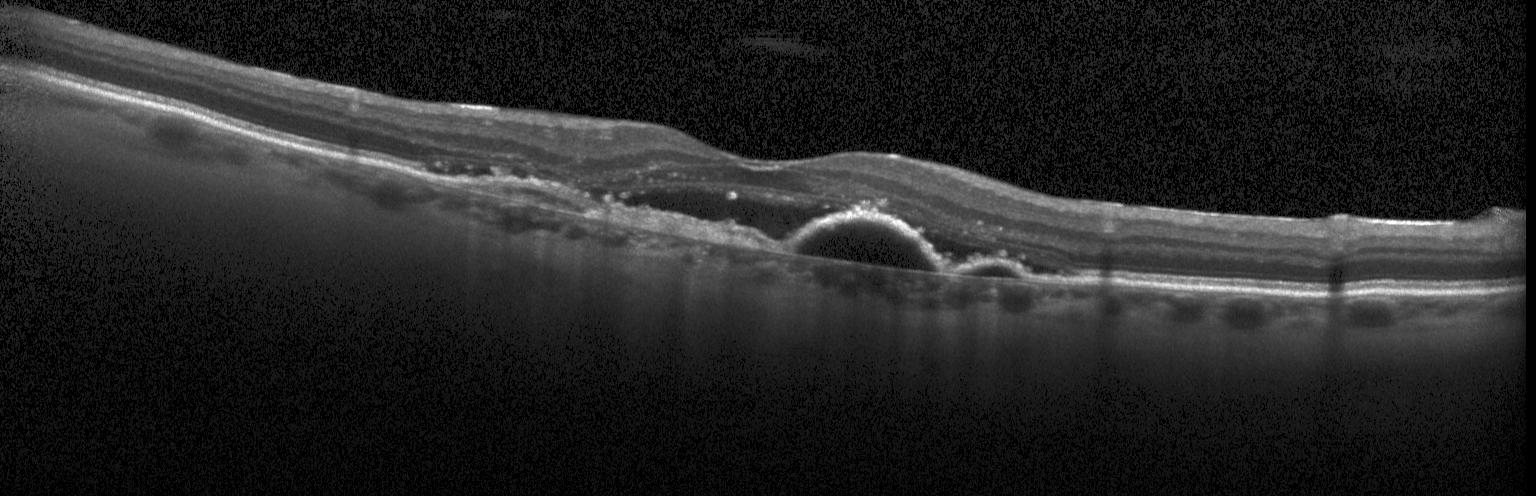

Retinal OCT cross-section · instrument: Heidelberg Spectralis — The scan shows a choroidal neovascular membrane.